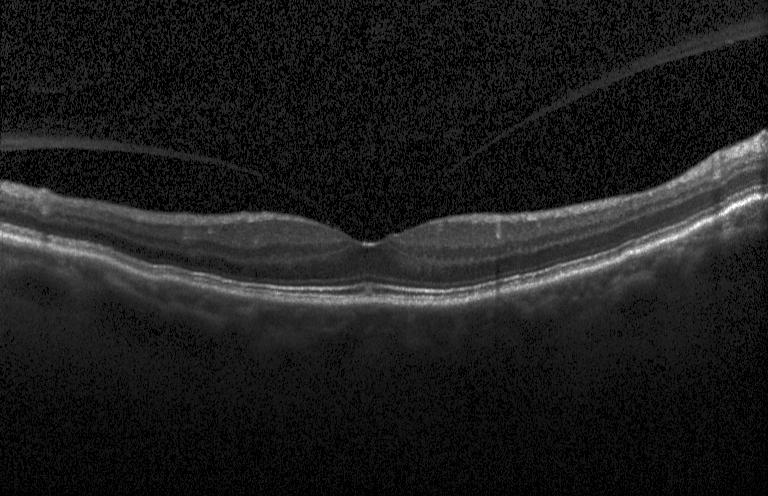
Optical coherence tomography B-scan
Diagnosis: no CNV, DME, or drusen.